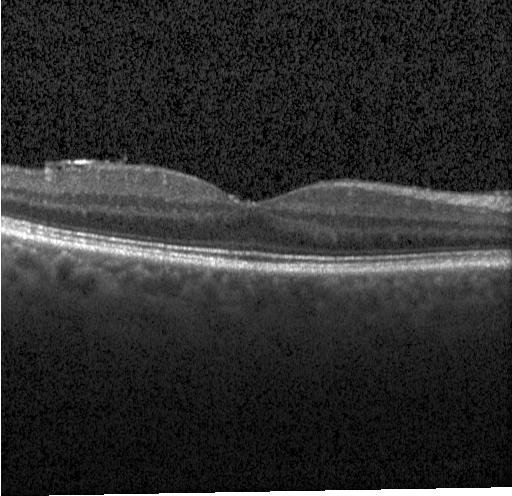
Acquired on a Heidelberg Spectralis · fovea-centered · OCT line scan
Neither choroidal neovascularization, diabetic macular edema, nor drusen.